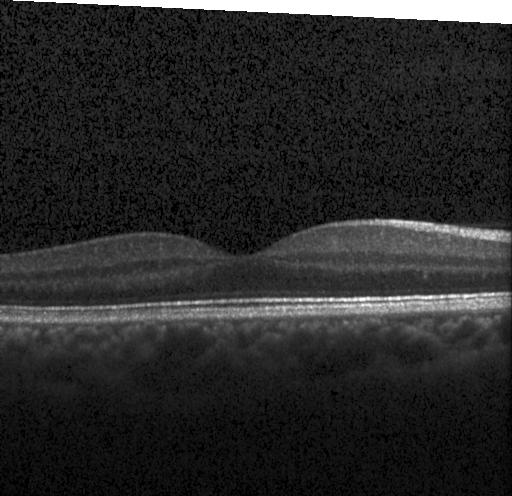 Spectral-domain OCT B-scan: neither choroidal neovascularization, diabetic macular edema, nor drusen.